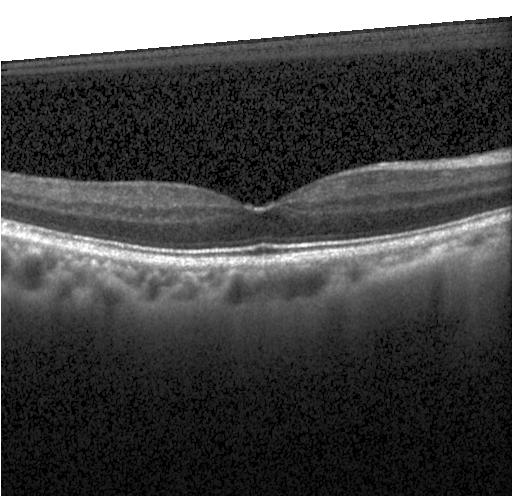

Assessment: neither choroidal neovascularization, diabetic macular edema, nor drusen.